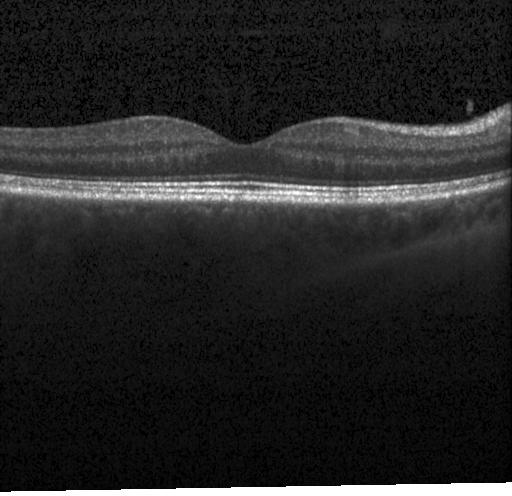
Spectral-domain optical coherence tomography; Heidelberg Spectralis; fovea-centered; OCT B-scan.
Macular OCT: no choroidal neovascularization, diabetic macular edema, or drusen.